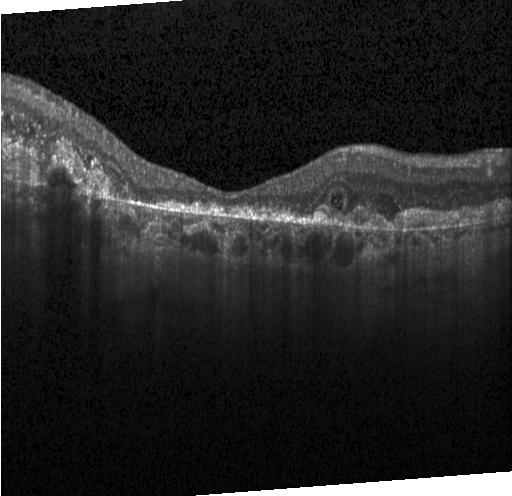 Spectral-domain OCT; optical coherence tomography scan — The scan shows a choroidal neovascular membrane.